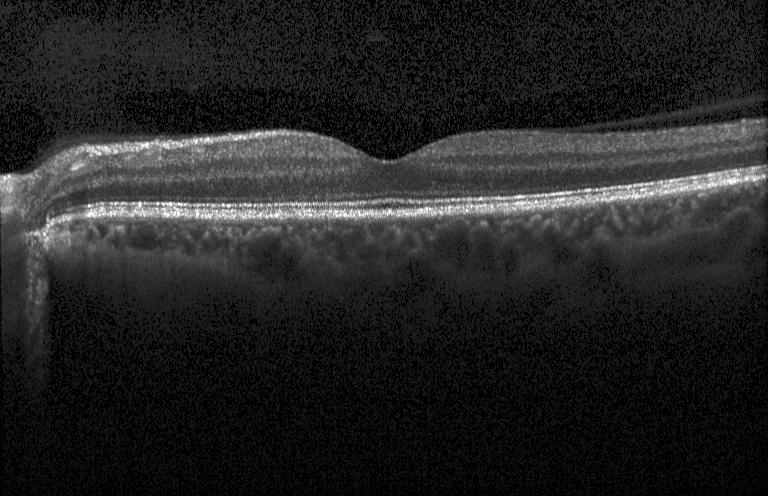
Retinal OCT B-scan. Impression: neither CNV, DME, nor drusen.